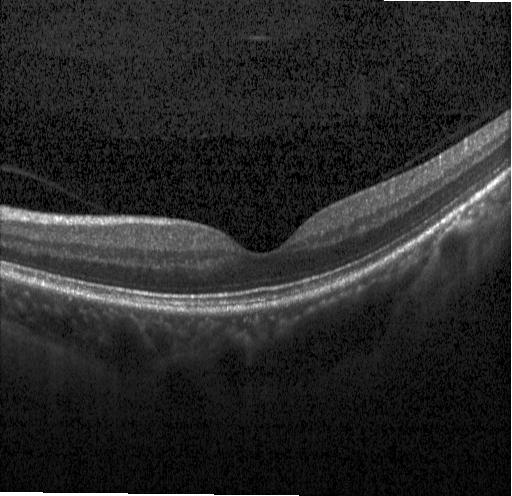 Retinal OCT cross-section — Neither choroidal neovascularization, diabetic macular edema, nor drusen.